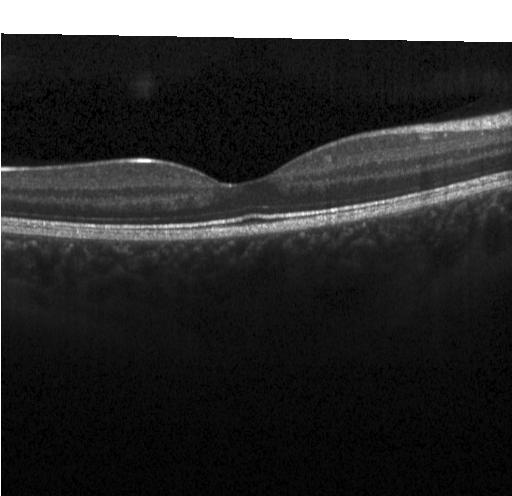 Impression: no evidence of choroidal neovascularization, diabetic macular edema, or drusen.